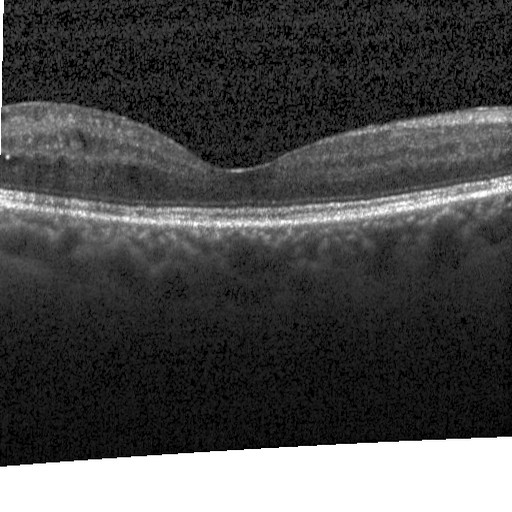

Diabetic macular edema.